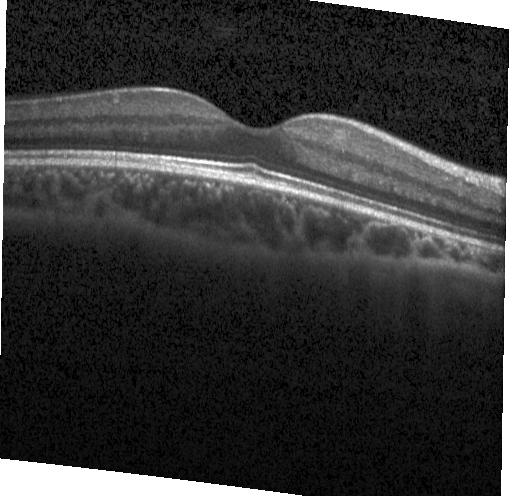

Dx: no choroidal neovascularization, diabetic macular edema, or drusen.